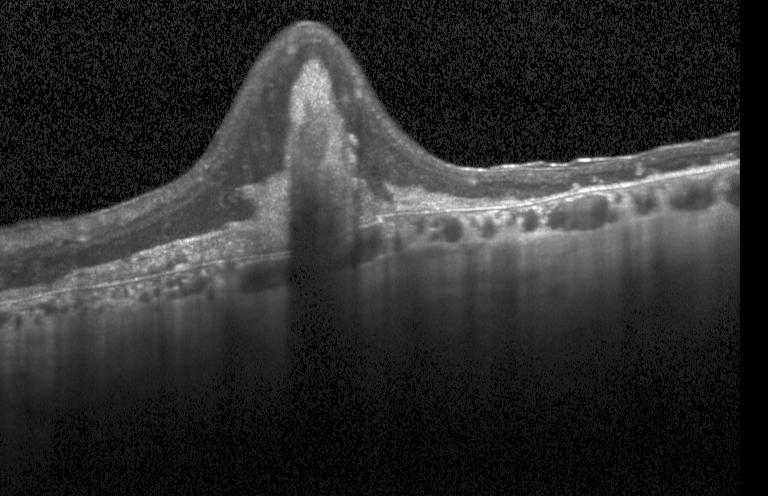
Macular OCT: a choroidal neovascular membrane.